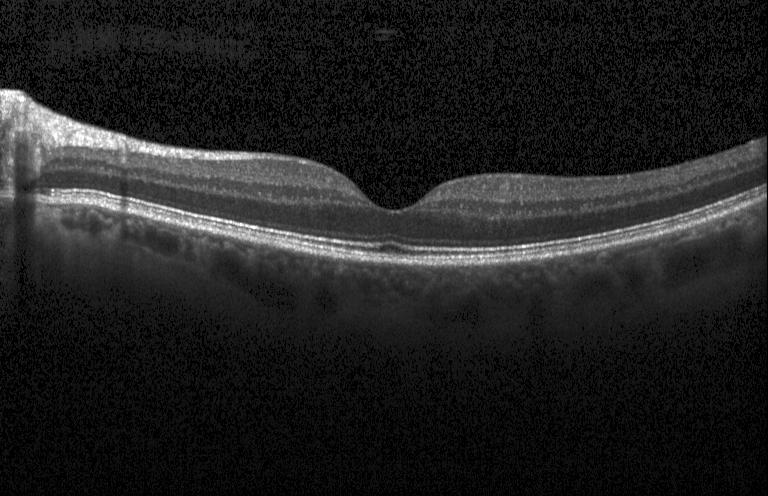

Retinal OCT B-scan, instrument: Heidelberg Spectralis. The scan shows no choroidal neovascularization, diabetic macular edema, or drusen.